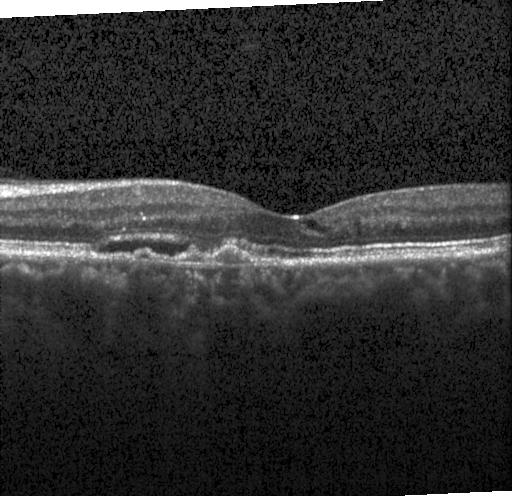
Retinal OCT B-scan; SD-OCT; through the macula.
Macular OCT: choroidal neovascularization.